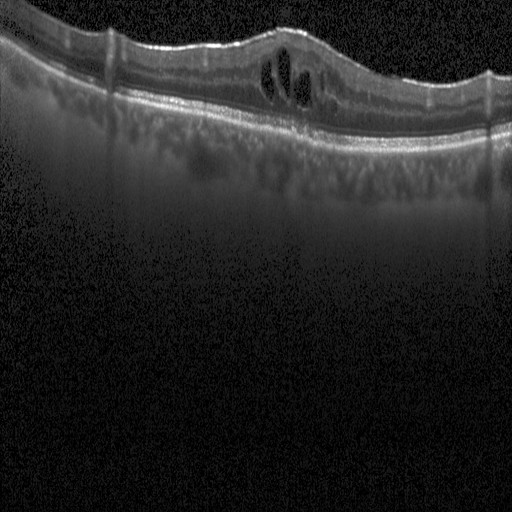
Heidelberg Spectralis OCT system. Macular scan. Spectral-domain OCT. Optical coherence tomography scan. Finding: diabetic macular edema.